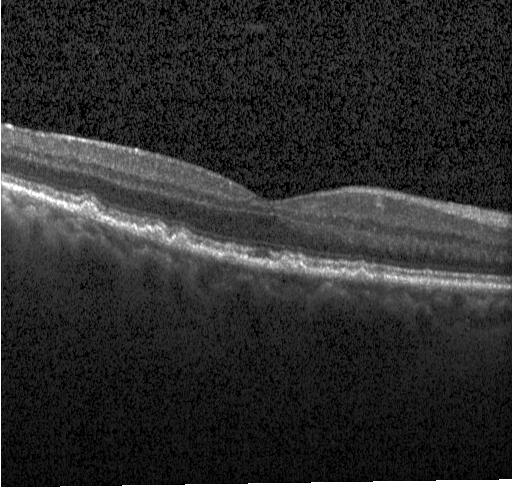

OCT line scan. Diagnosis: sub-RPE drusenoid deposits.